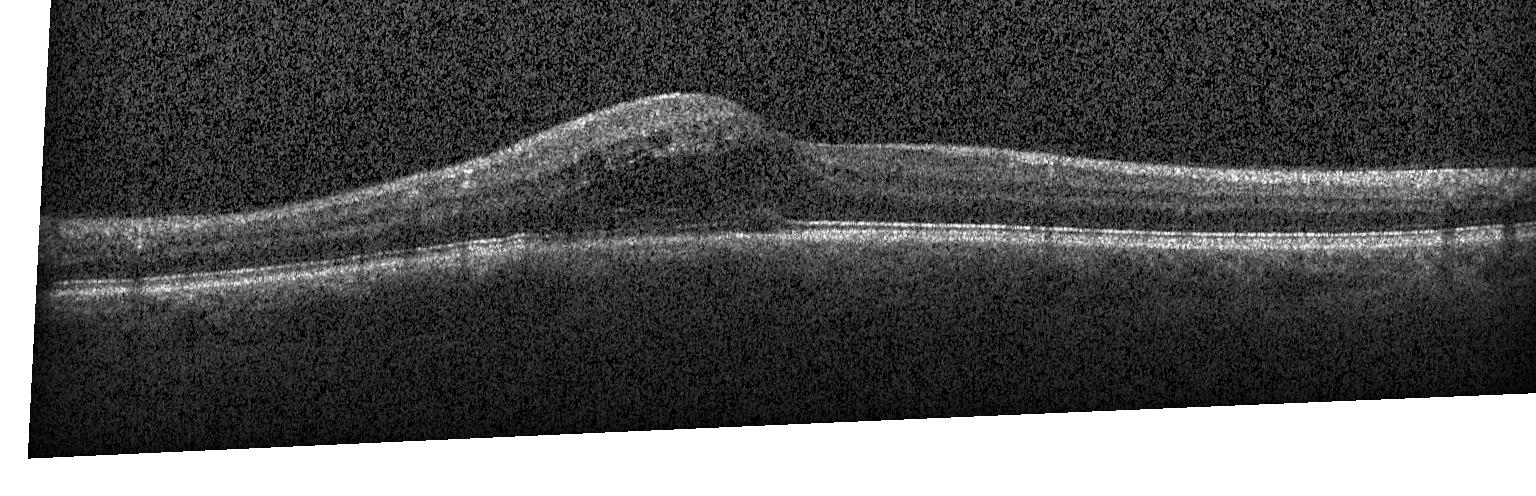
Optical coherence tomography B-scan. Assessment: diabetic macular edema (DME).